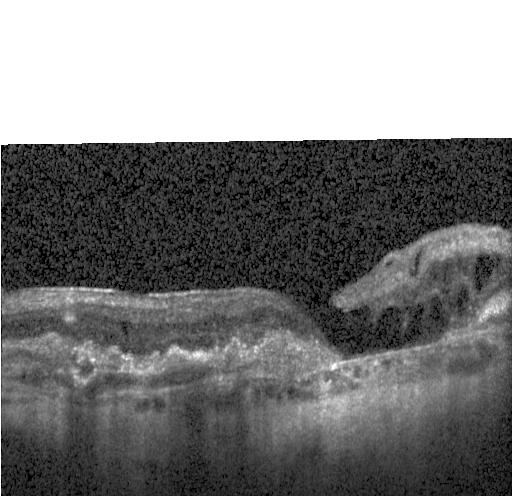
Optical coherence tomography scan
Diagnosis: choroidal neovascularization (CNV).